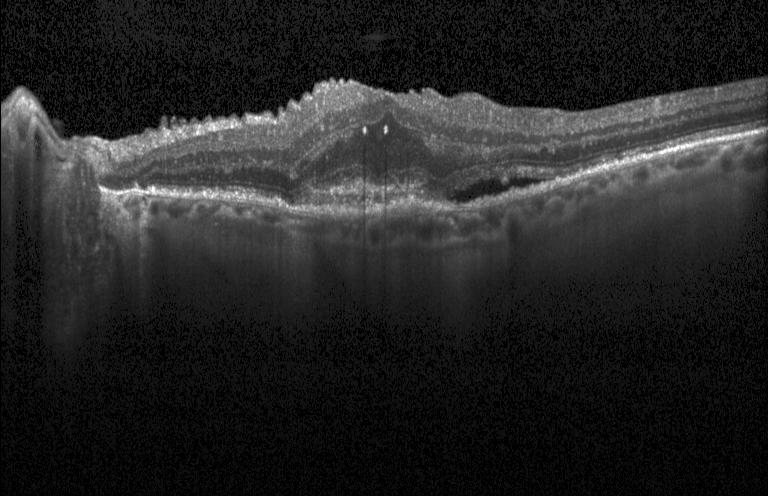

Impression: a choroidal neovascular membrane.